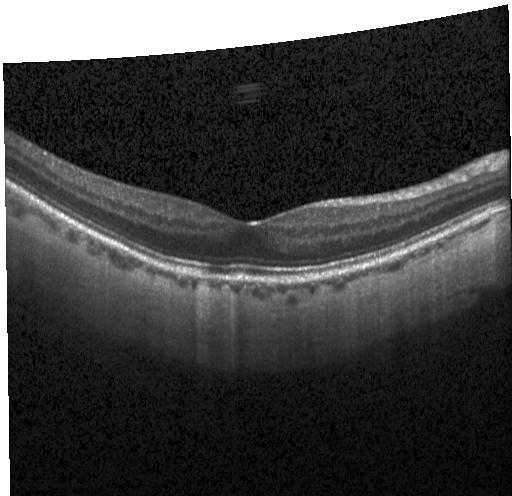 Optical coherence tomography B-scan. The scan shows neither choroidal neovascularization, diabetic macular edema, nor drusen.